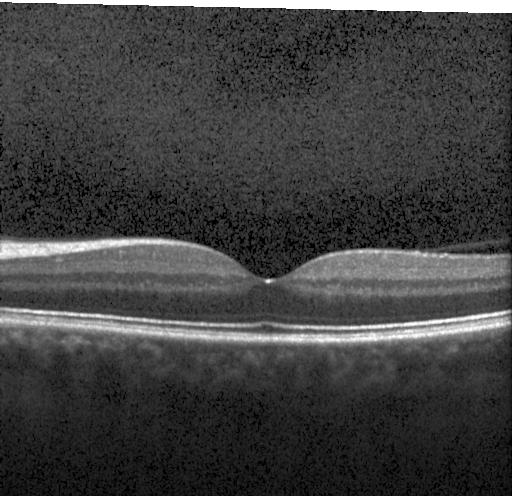 Macular scan; OCT B-scan. Assessment: no choroidal neovascularization, diabetic macular edema, or drusen.